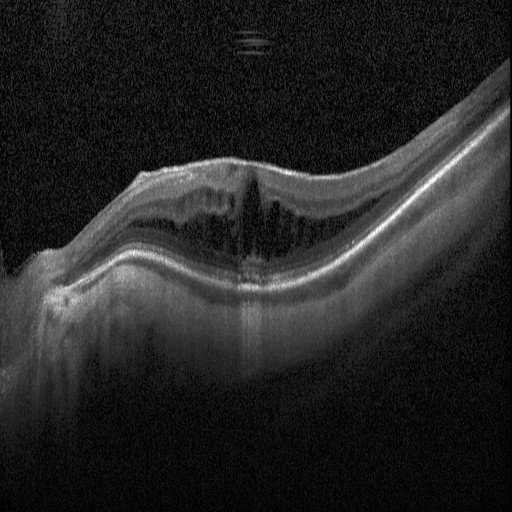

DME.